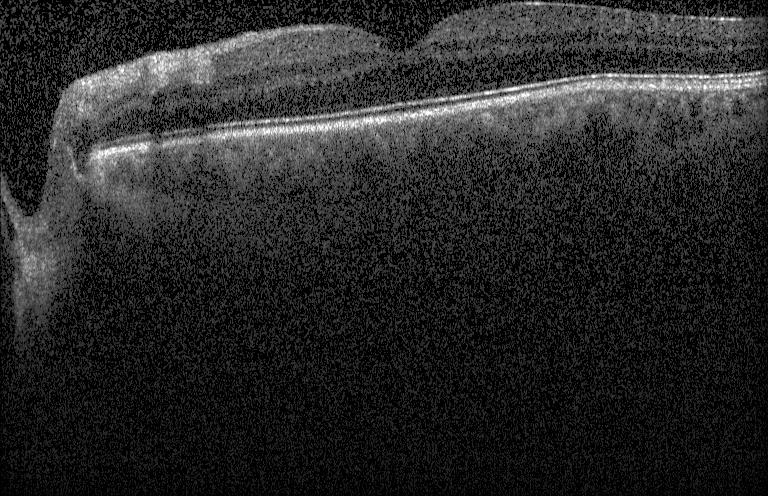

Finding: no choroidal neovascularization, no diabetic macular edema, and no drusen.